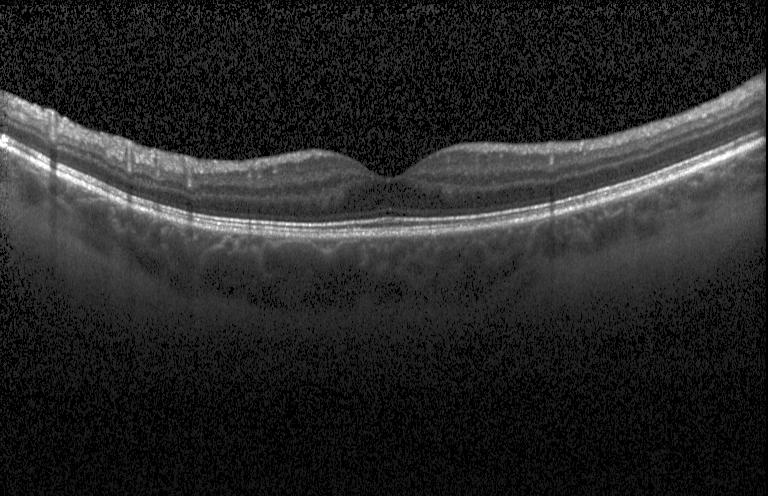 Optical coherence tomography scan. Finding: neither choroidal neovascularization, diabetic macular edema, nor drusen.